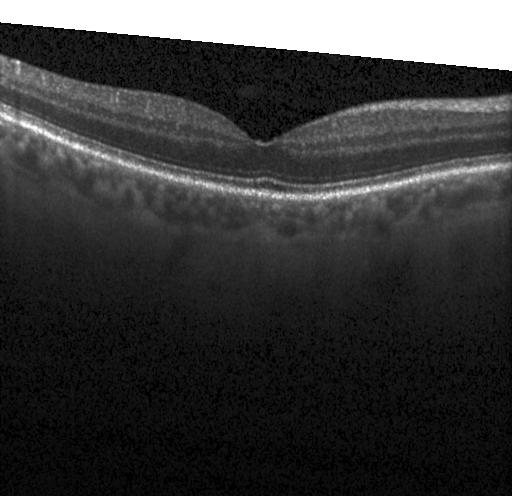
The scan shows no CNV, no DME, and no drusen.